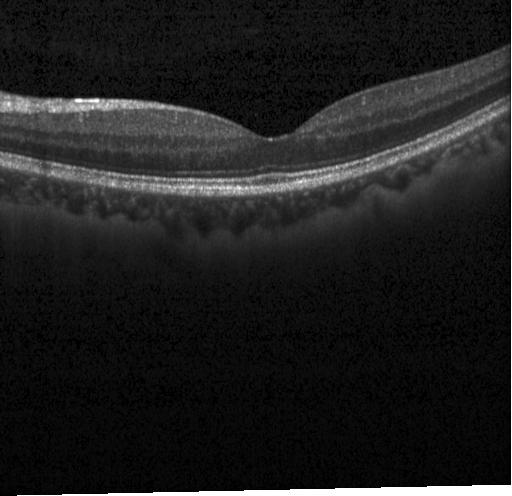
Spectral-domain OCT B-scan: neither CNV, DME, nor drusen.